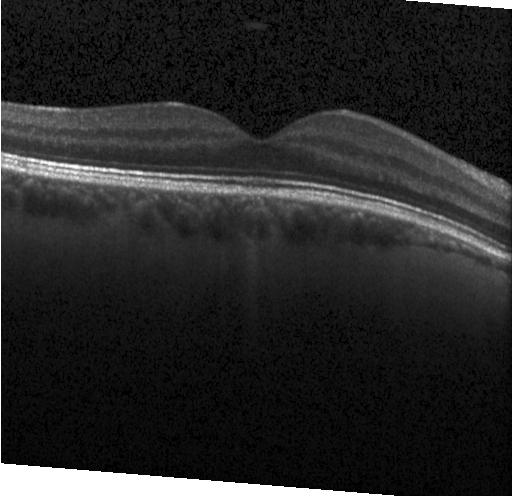

Heidelberg Spectralis OCT system; optical coherence tomography B-scan. Neither CNV, DME, nor drusen.